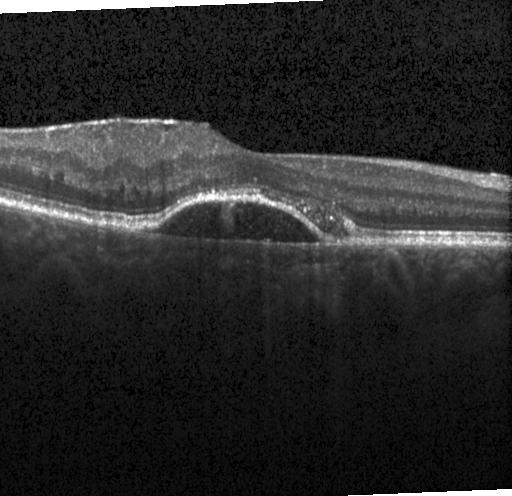 Spectral-domain OCT, optical coherence tomography B-scan, fovea-centered
This B-scan demonstrates choroidal neovascularization (CNV).